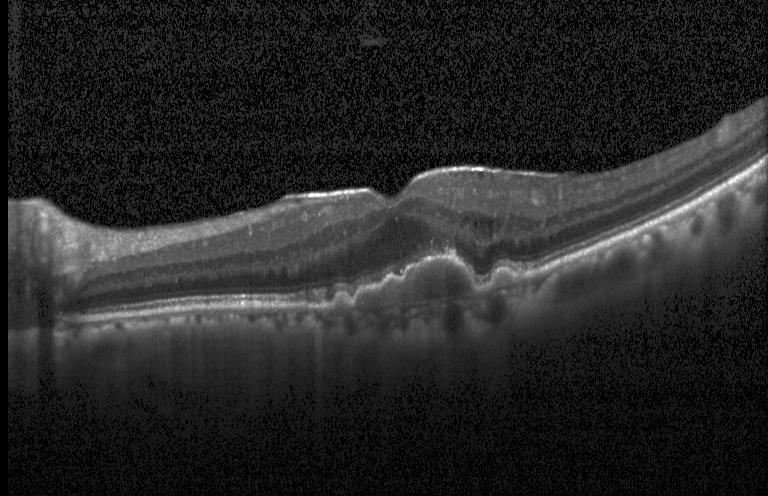
Optical coherence tomography scan; spectral-domain optical coherence tomography; Heidelberg Spectralis OCT system
Diagnosis: a choroidal neovascular membrane.